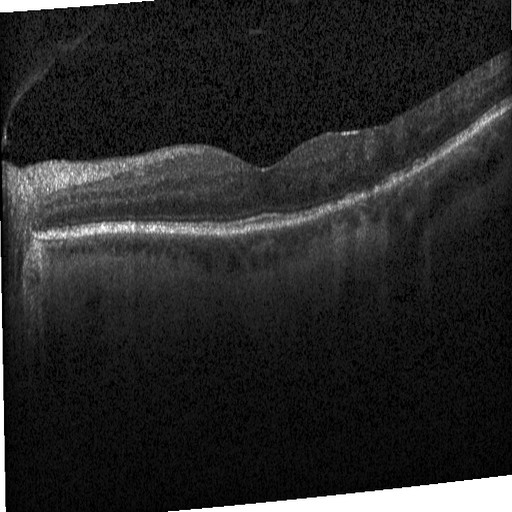
Diagnosis: DME.